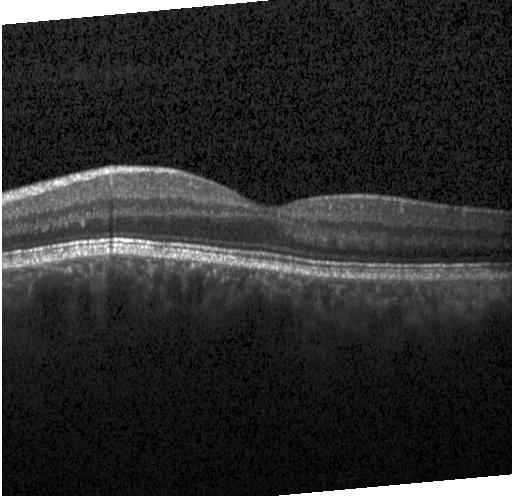 Centered on the fovea; Heidelberg Spectralis; OCT B-scan. Impression: no choroidal neovascularization, diabetic macular edema, or drusen.